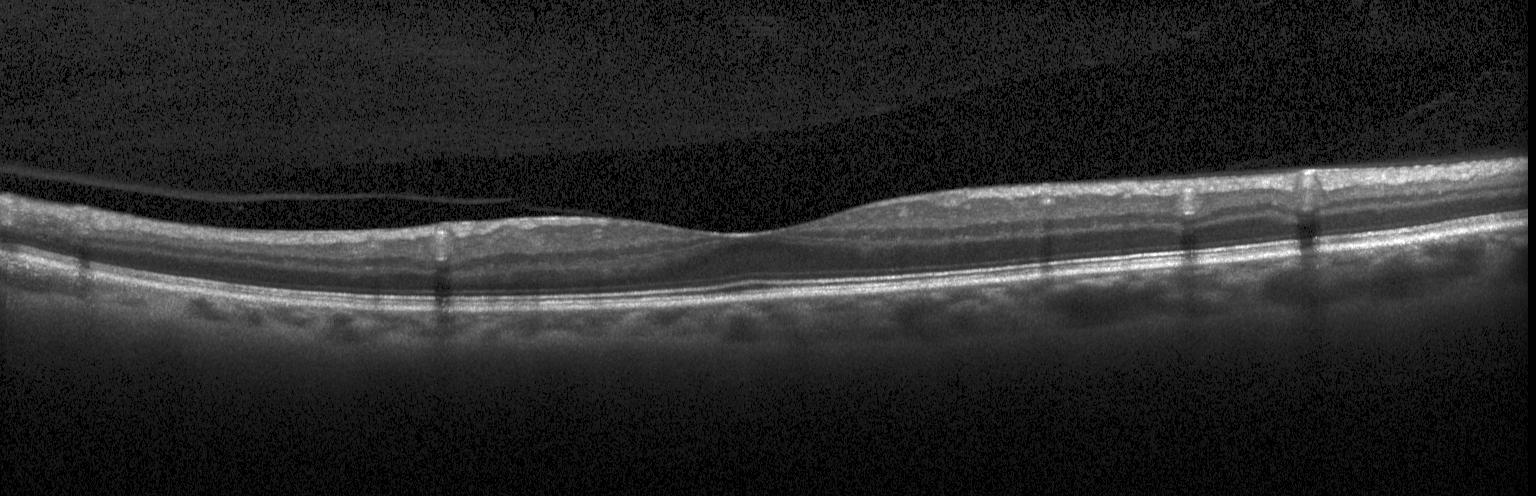 Assessment: neither choroidal neovascularization, diabetic macular edema, nor drusen.